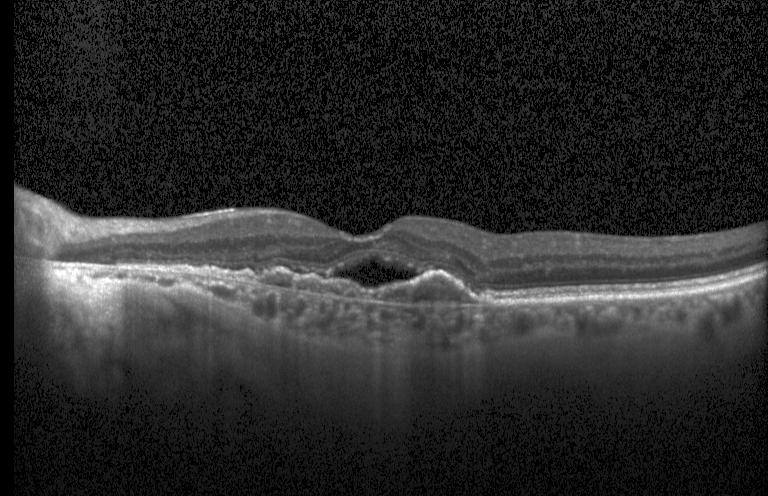 Heidelberg Spectralis OCT system · macular scan · OCT line scan · spectral-domain optical coherence tomography. Impression: a choroidal neovascular membrane.